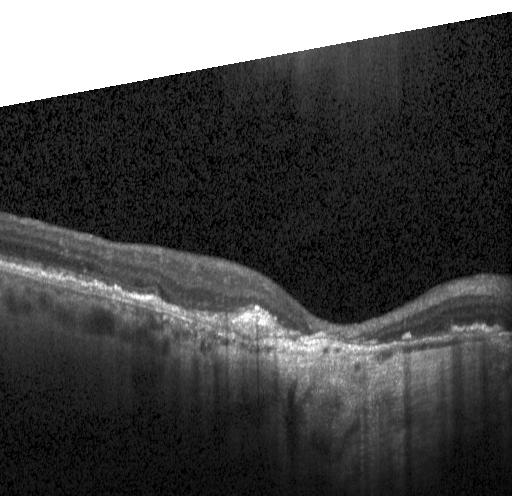 Macular OCT: a choroidal neovascular membrane.